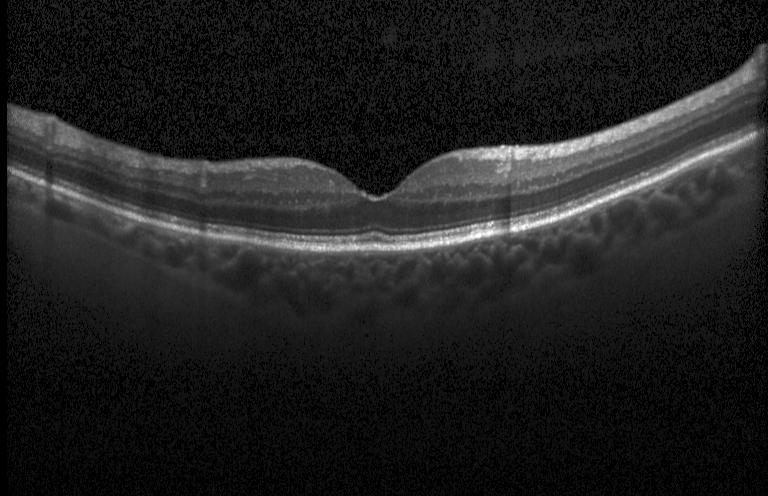

Spectral-domain OCT. Heidelberg Spectralis. Fovea-centered. OCT line scan
Assessment: no CNV, DME, or drusen.